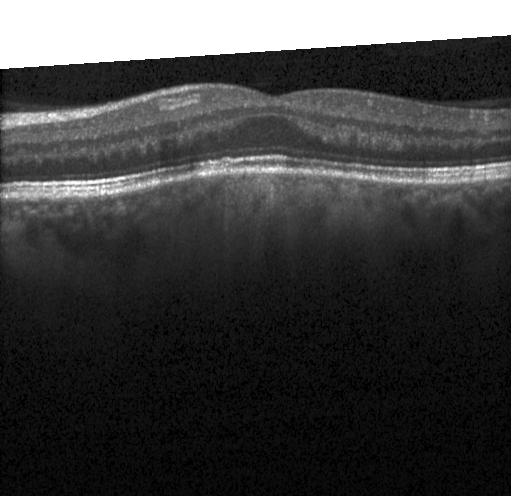

The scan shows no choroidal neovascularization, no diabetic macular edema, and no drusen.